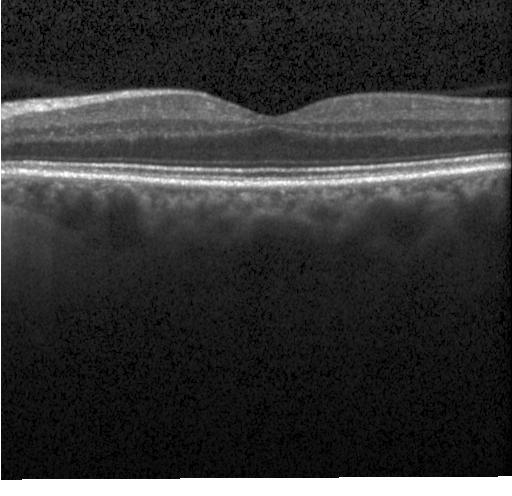 OCT scan showing no choroidal neovascularization, no diabetic macular edema, and no drusen.